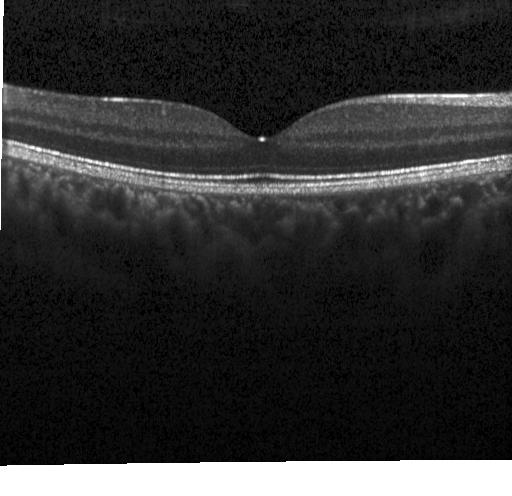

OCT finding: neither CNV, DME, nor drusen.